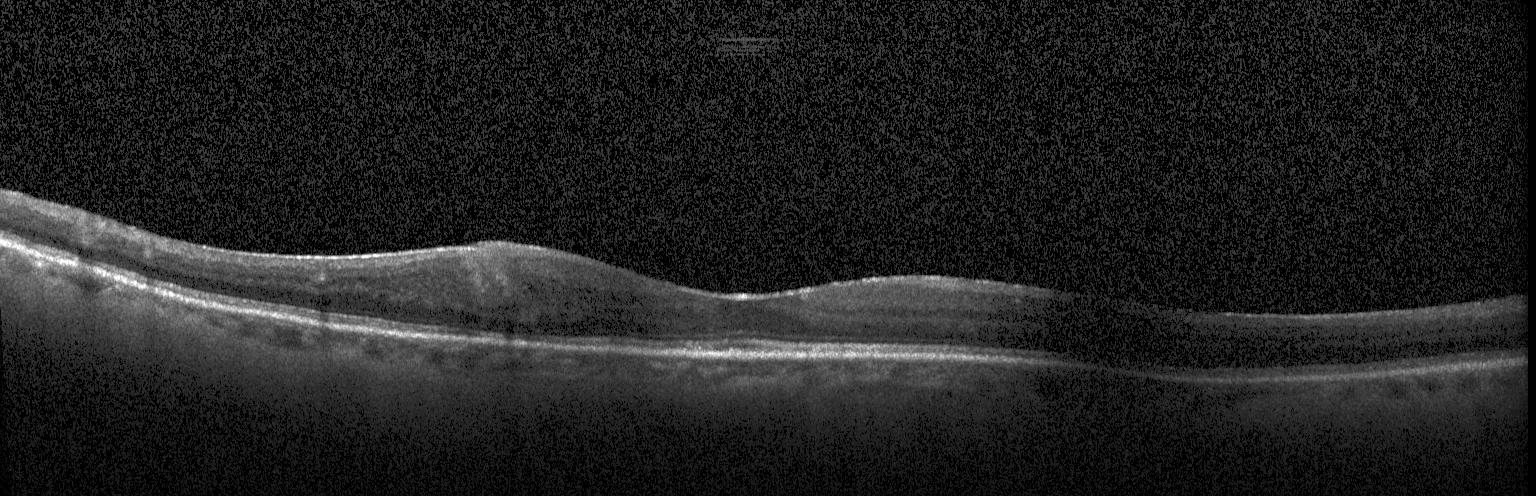 Optical coherence tomography B-scan — This B-scan demonstrates no CNV, DME, or drusen.